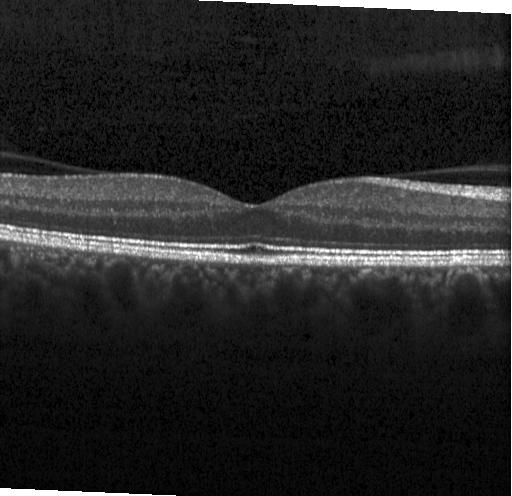
OCT finding: no CNV, DME, or drusen.